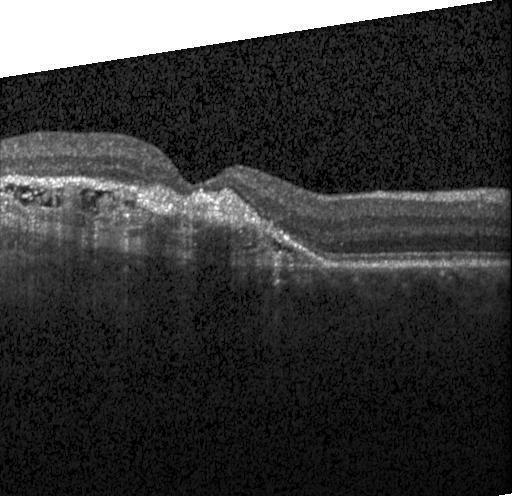

OCT finding: a choroidal neovascular membrane.